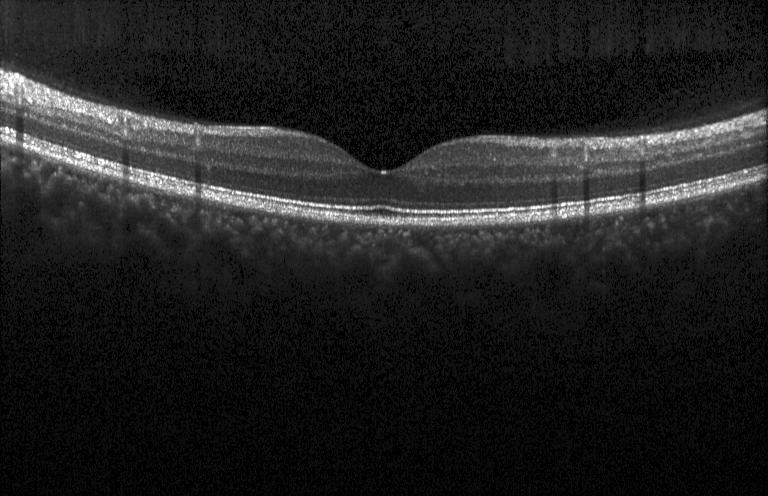 Impression: no CNV, DME, or drusen.